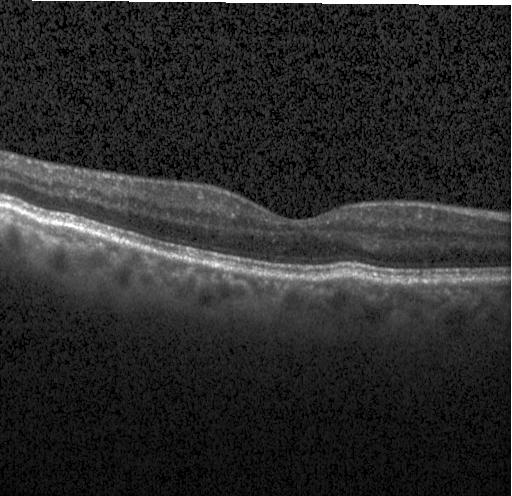

OCT line scan. No choroidal neovascularization, diabetic macular edema, or drusen.